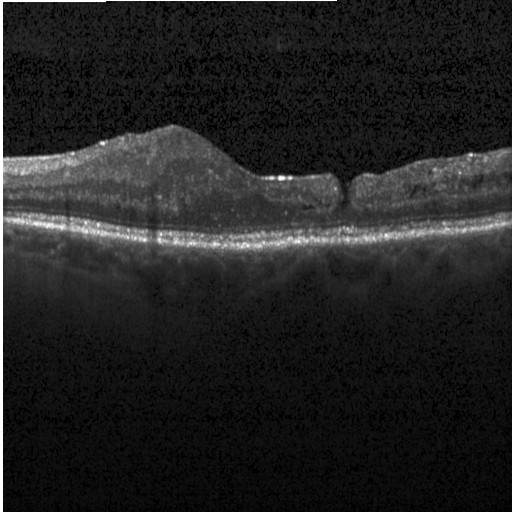 Retinal OCT cross-section.
Macular OCT: DME.